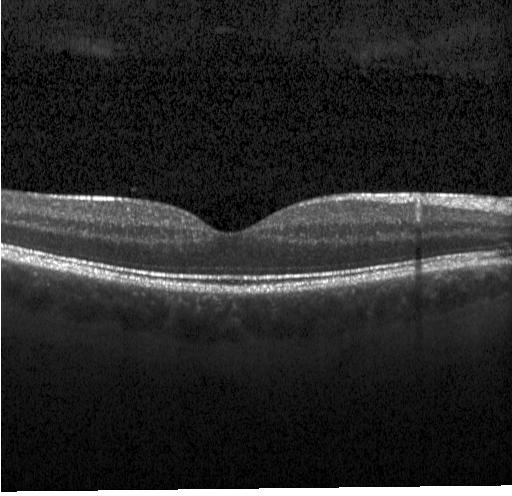

OCT finding: no choroidal neovascularization, diabetic macular edema, or drusen.